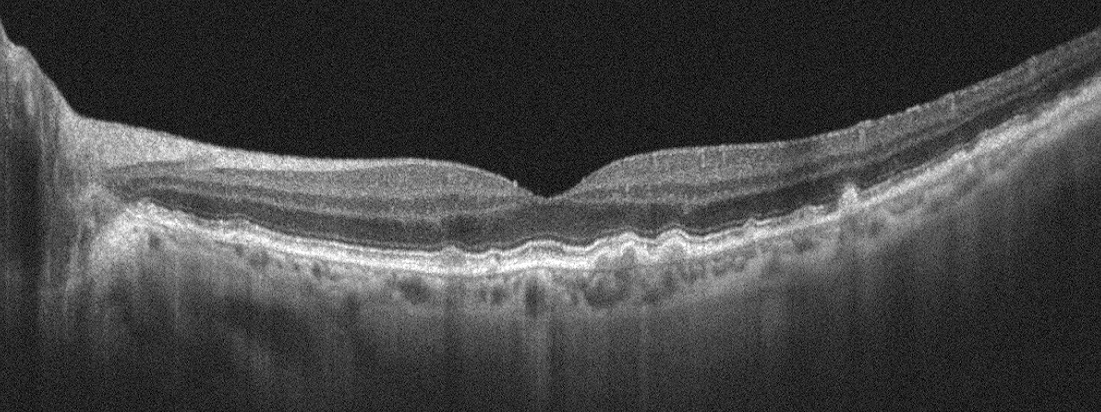
The scan shows age-related macular degeneration.